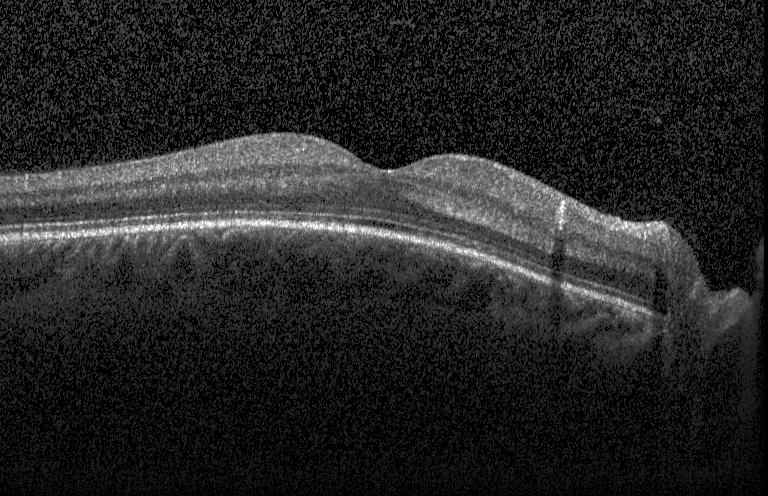

Retinal OCT cross-section
Impression: no evidence of choroidal neovascularization, diabetic macular edema, or drusen.